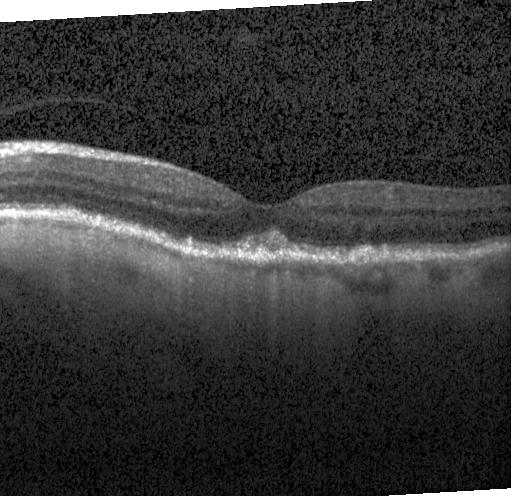 OCT line scan, Heidelberg Spectralis. Multiple drusen.